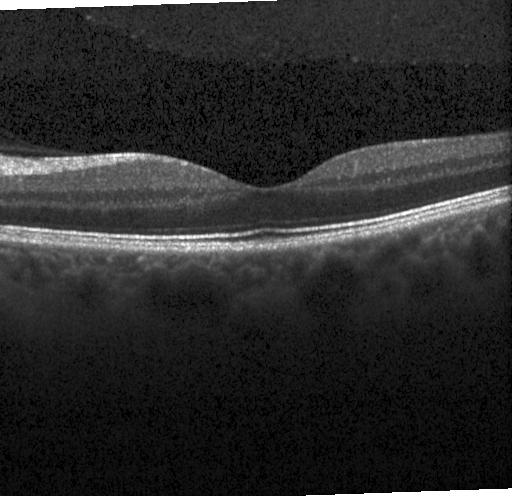

Through the macula, spectral-domain OCT, instrument: Heidelberg Spectralis, retinal OCT cross-section
This B-scan demonstrates no choroidal neovascularization, no diabetic macular edema, and no drusen.